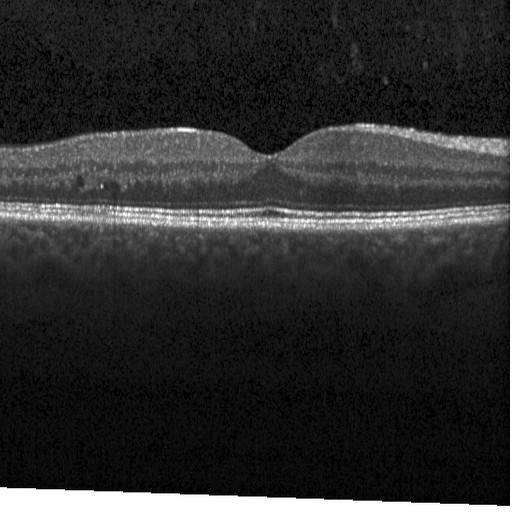
Finding: diabetic macular edema (DME).